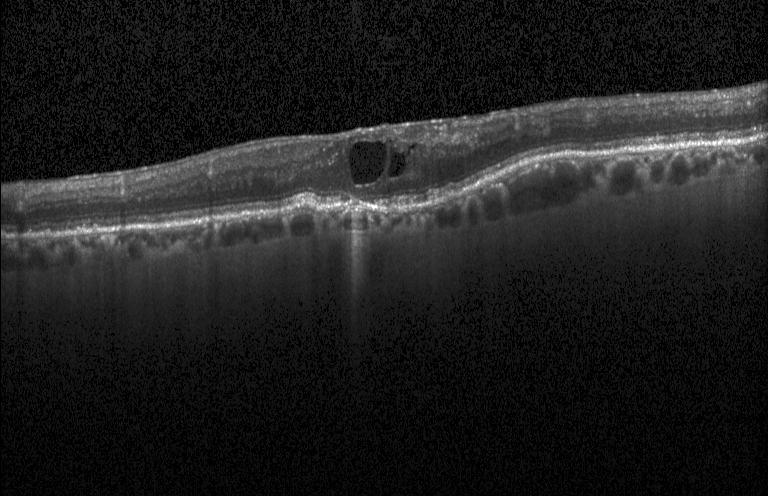

Impression: a choroidal neovascular membrane.